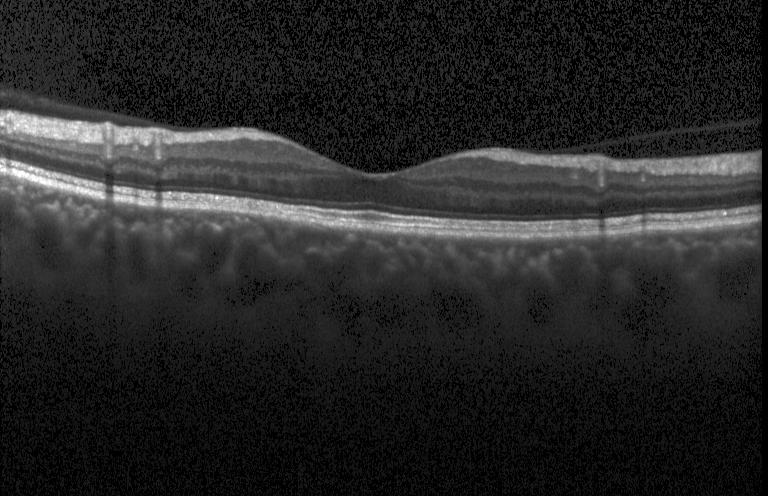
Impression: no choroidal neovascularization, no diabetic macular edema, and no drusen.